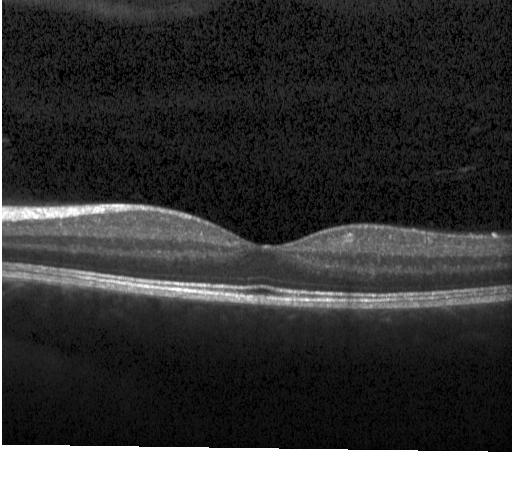

Macular scan · OCT B-scan · spectral-domain optical coherence tomography · instrument: Heidelberg Spectralis. This B-scan demonstrates no evidence of CNV, DME, or drusen.